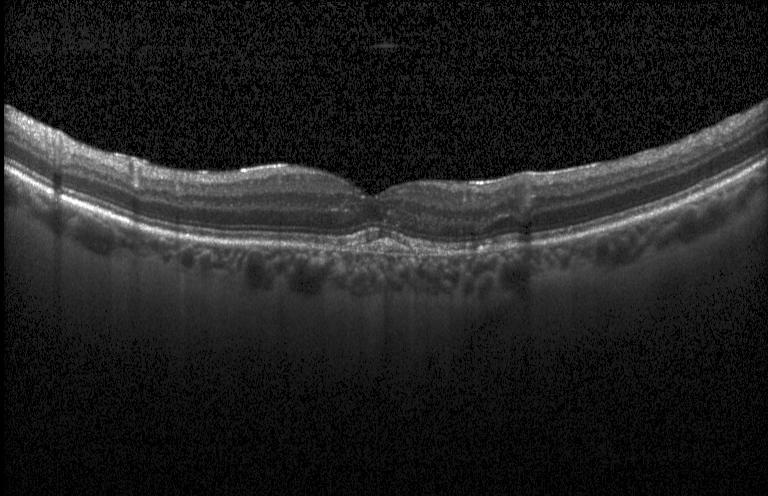
Heidelberg Spectralis OCT system. Spectral-domain OCT. Horizontal scan through the fovea. OCT B-scan — CNV.